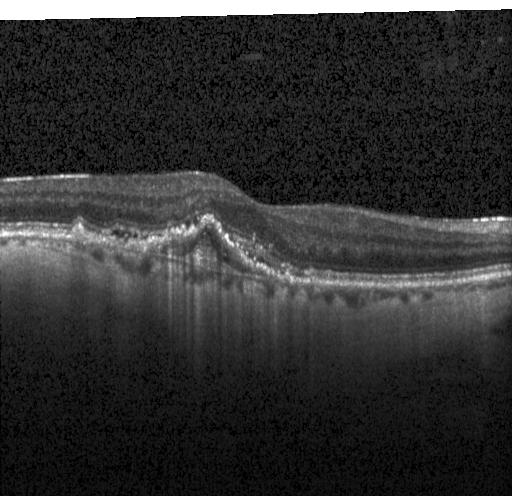

Macular OCT: choroidal neovascularization (CNV).